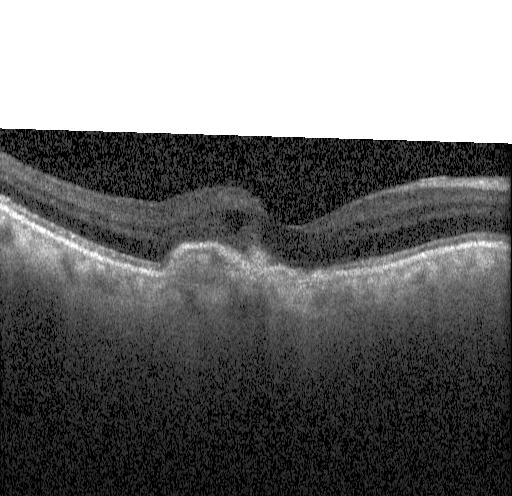
Macular OCT demonstrating CNV.